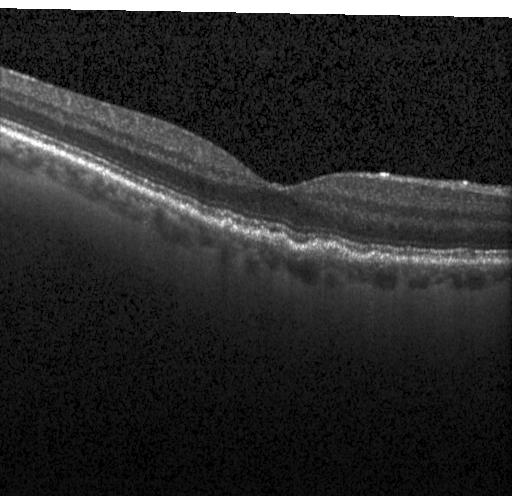
OCT line scan. Diagnosis: sub-RPE drusenoid deposits.